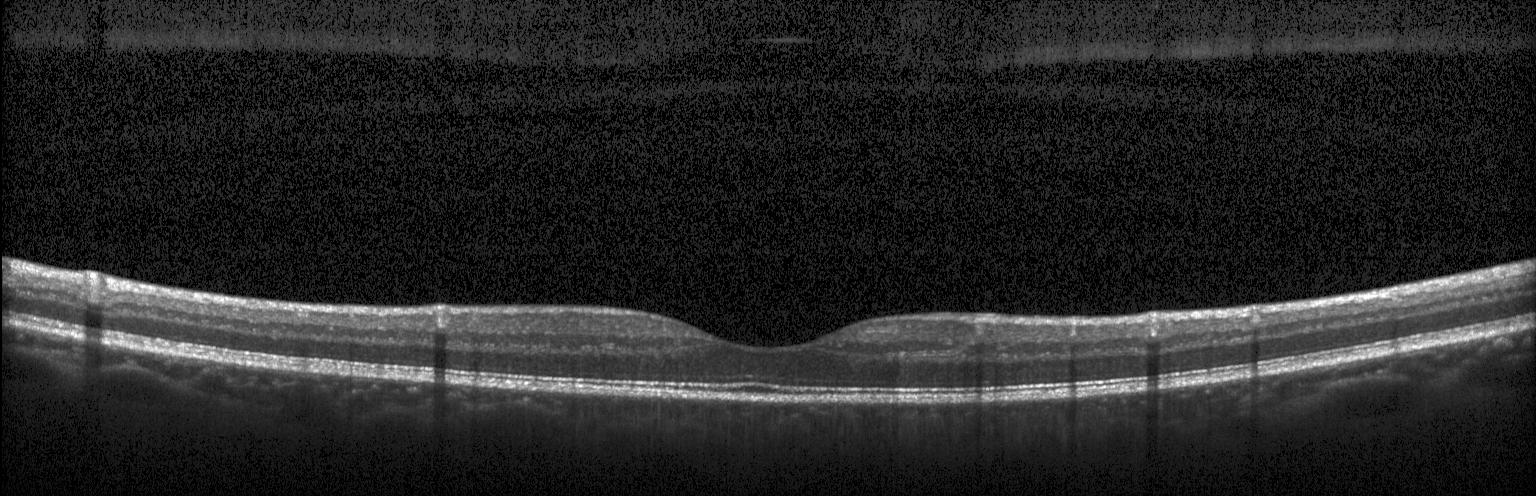
Retinal OCT cross-section. Impression: neither choroidal neovascularization, diabetic macular edema, nor drusen.